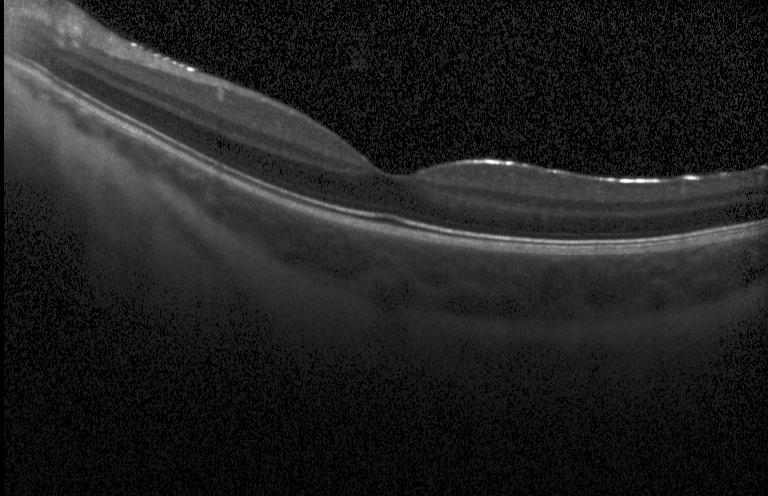

Centered on the fovea, SD-OCT, OCT B-scan
Impression: no evidence of choroidal neovascularization, diabetic macular edema, or drusen.